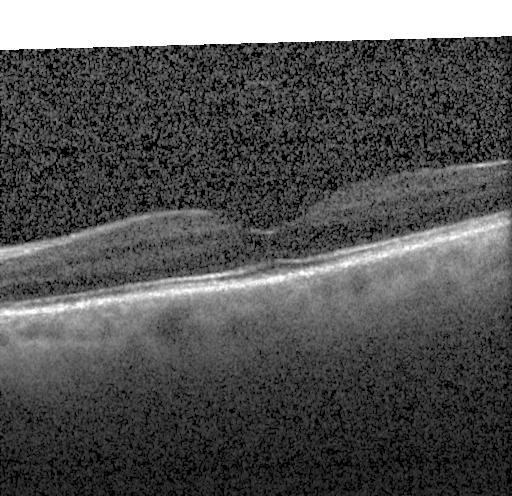 Spectral-domain OCT B-scan: neither choroidal neovascularization, diabetic macular edema, nor drusen.